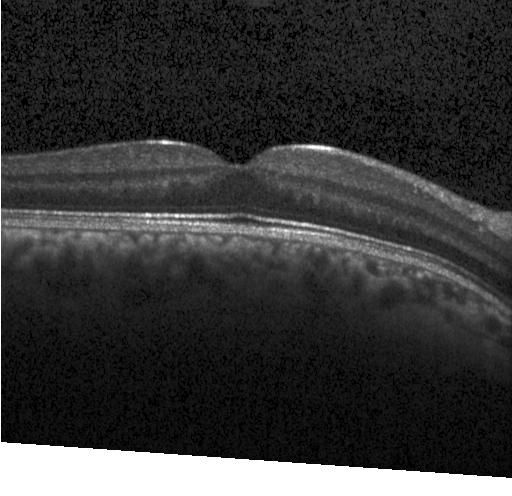

Finding: no choroidal neovascularization, no diabetic macular edema, and no drusen.